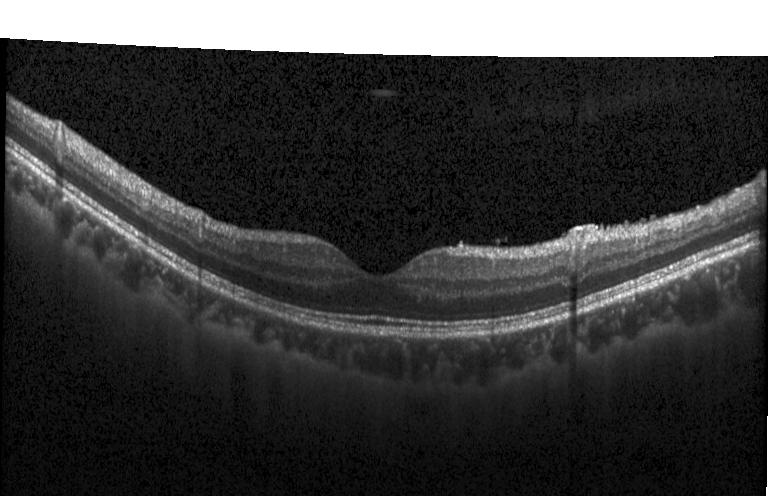
Dx: no choroidal neovascularization, no diabetic macular edema, and no drusen.